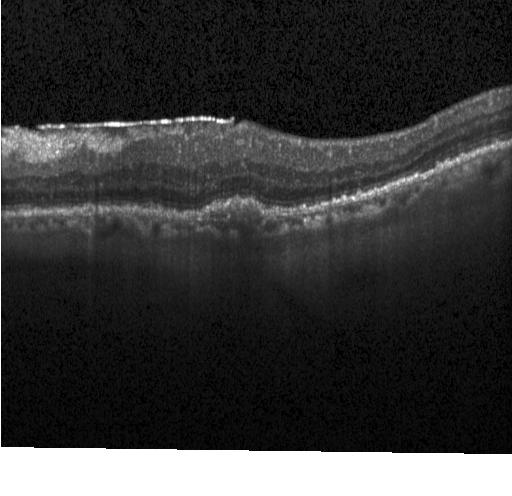 OCT line scan — Diagnosis: a choroidal neovascular membrane.